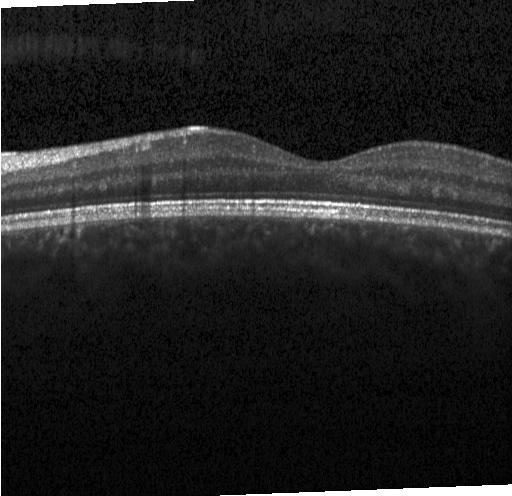

Fovea-centered, optical coherence tomography scan, spectral-domain optical coherence tomography — This B-scan demonstrates no choroidal neovascularization, diabetic macular edema, or drusen.